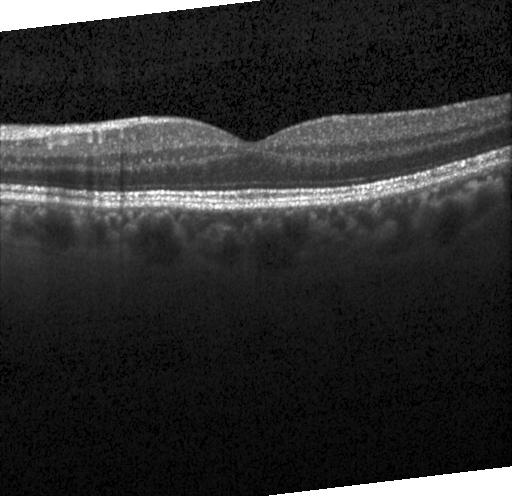 Macular scan; OCT B-scan
OCT finding: no evidence of CNV, DME, or drusen.